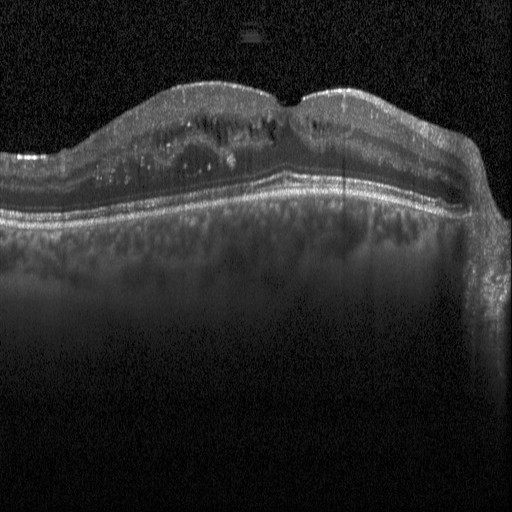 Diagnosis: DME.